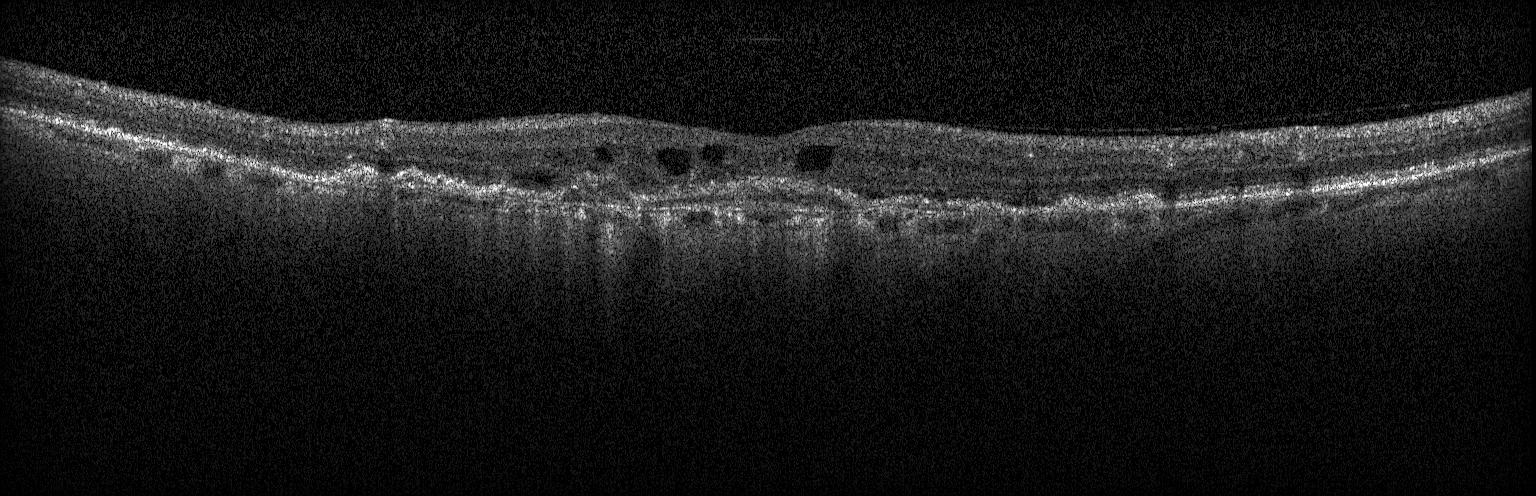
Horizontal scan through the fovea; optical coherence tomography B-scan; Heidelberg Spectralis OCT system. Finding: choroidal neovascularization (CNV).